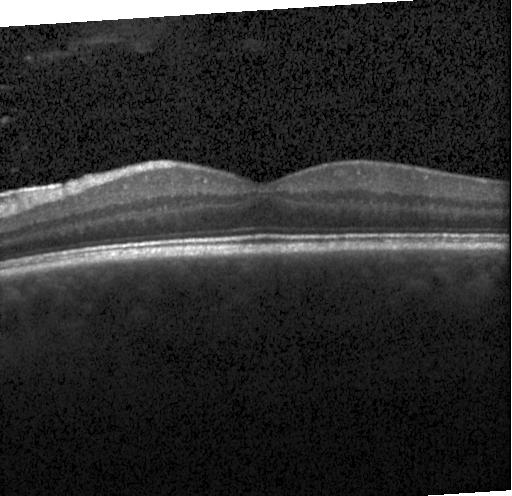
OCT scan showing neither CNV, DME, nor drusen.